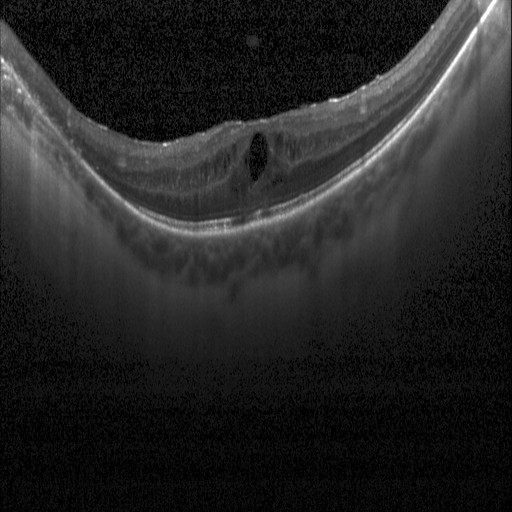
Instrument: Heidelberg Spectralis, retinal OCT cross-section, fovea-centered, spectral-domain OCT
This B-scan demonstrates DME.